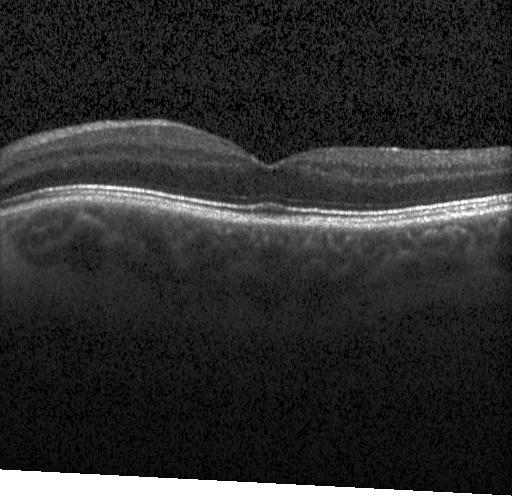
Impression: neither choroidal neovascularization, diabetic macular edema, nor drusen.